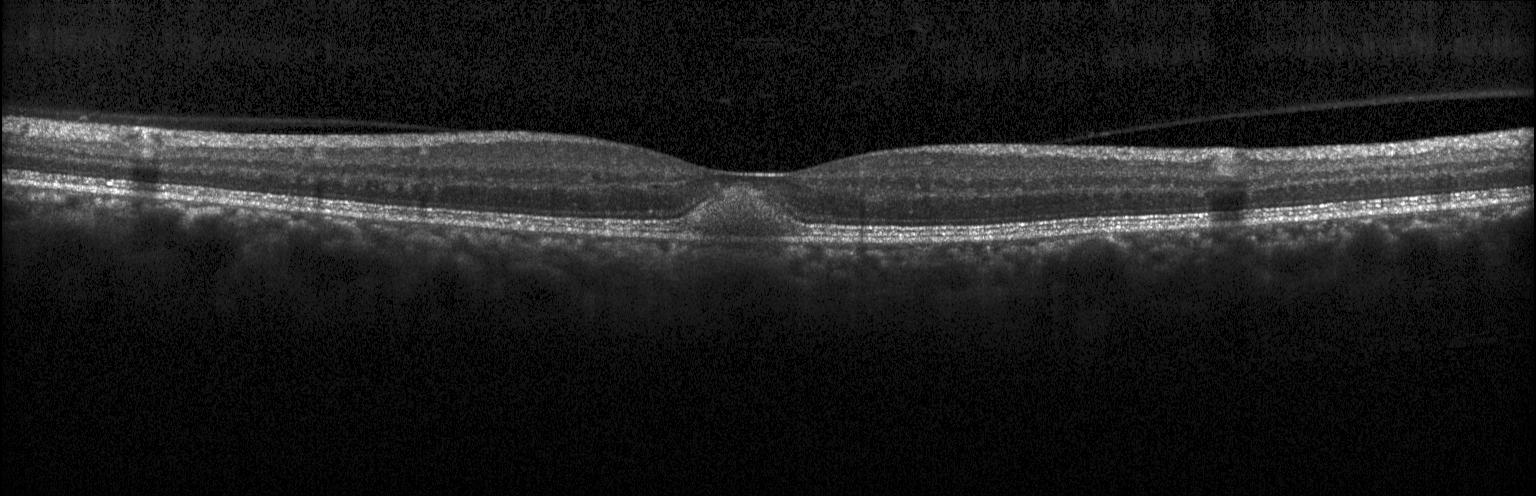
Optical coherence tomography B-scan. Macular OCT: CNV.